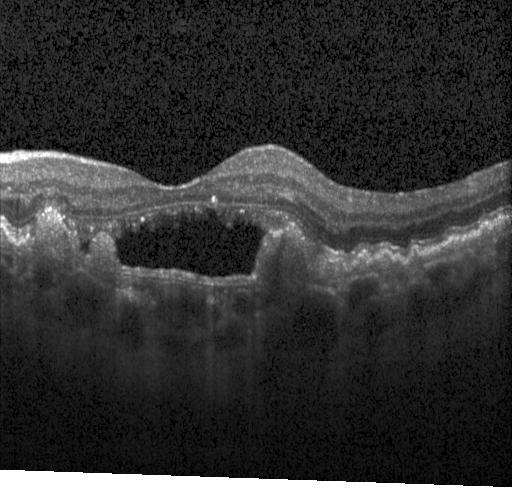 Diagnosis: choroidal neovascularization (CNV).